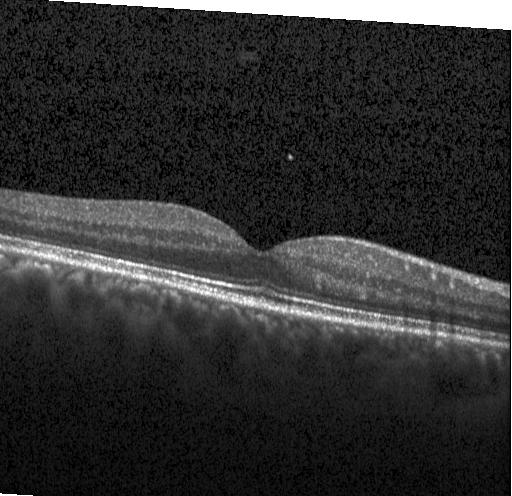
Impression: neither choroidal neovascularization, diabetic macular edema, nor drusen.